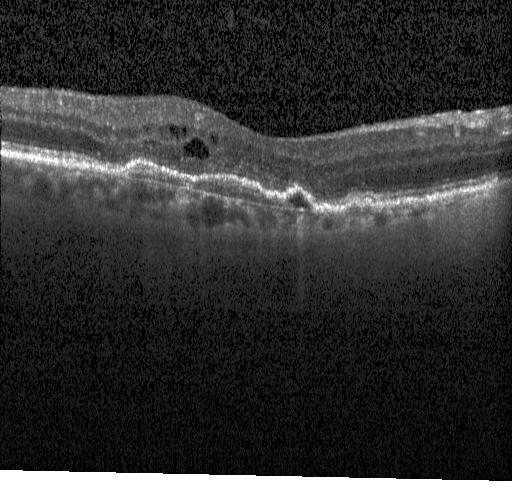

Macular OCT demonstrating a choroidal neovascular membrane.